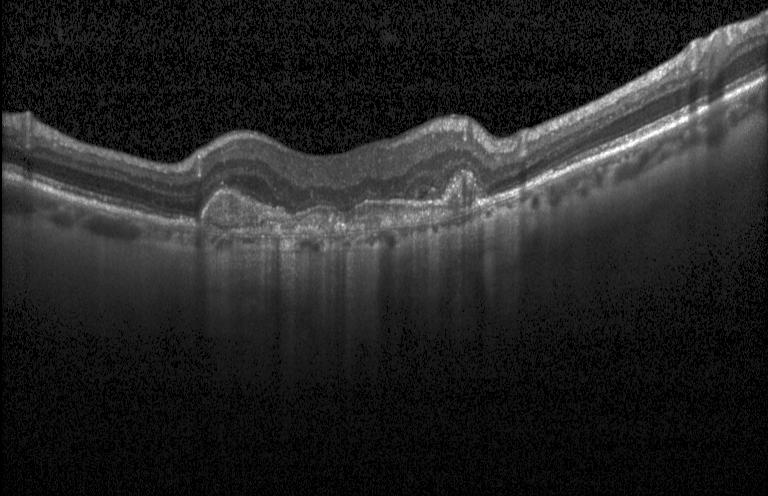 Retinal OCT cross-section. Macular scan. SD-OCT — The scan shows choroidal neovascularization.